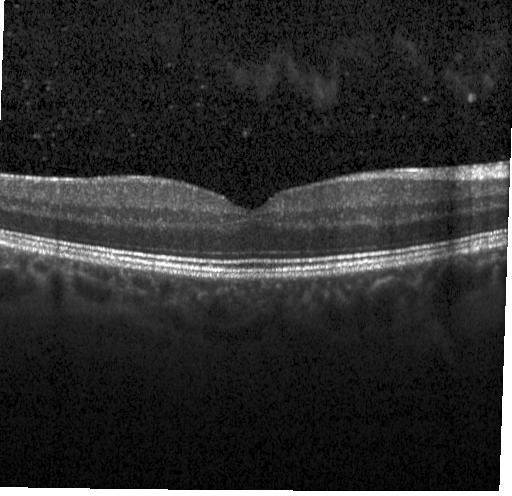
OCT line scan.
This B-scan demonstrates no evidence of choroidal neovascularization, diabetic macular edema, or drusen.